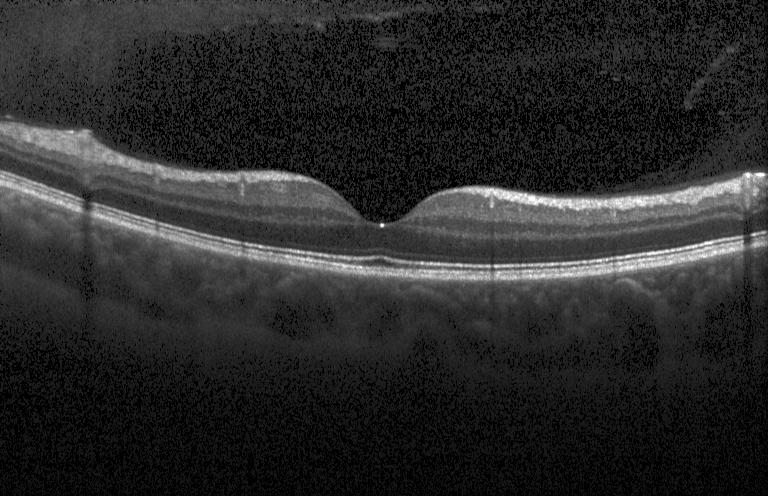

SD-OCT. Optical coherence tomography scan — Finding: no CNV, no DME, and no drusen.